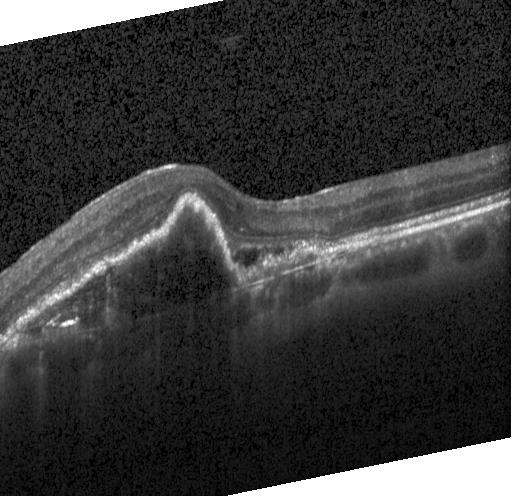
Retinal OCT cross-section · spectral-domain optical coherence tomography · through the macula · Heidelberg Spectralis OCT system.
Assessment: choroidal neovascularization.